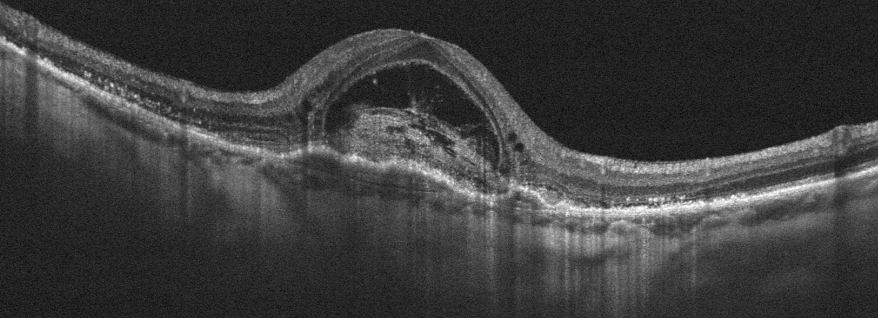
OCT line scan. OCT finding: AMD.